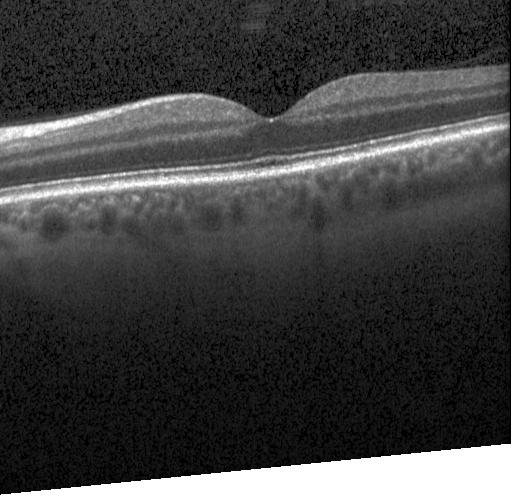 Spectral-domain OCT B-scan: no evidence of choroidal neovascularization, diabetic macular edema, or drusen.